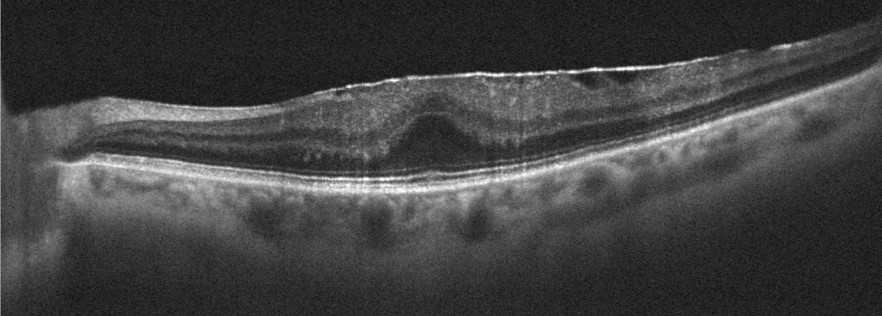 Spectral-domain OCT B-scan: epiretinal membrane (ERM).